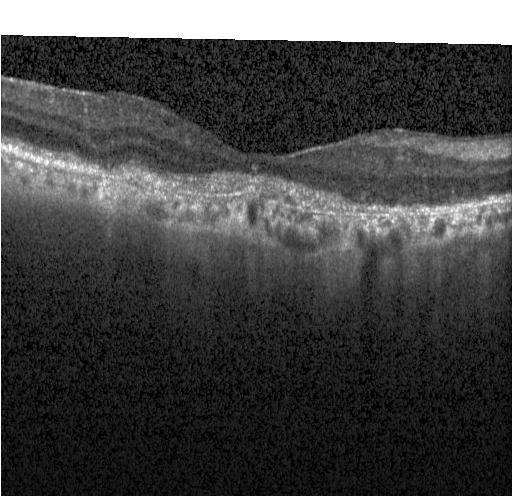

OCT scan showing a choroidal neovascular membrane.